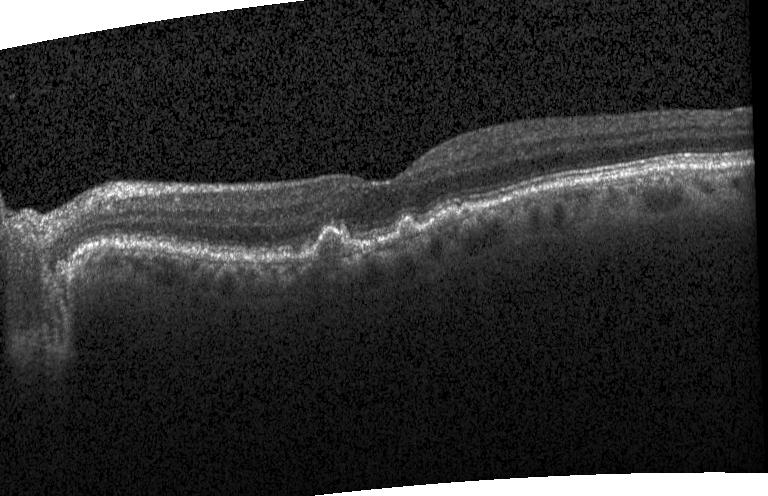
Assessment: multiple drusen.